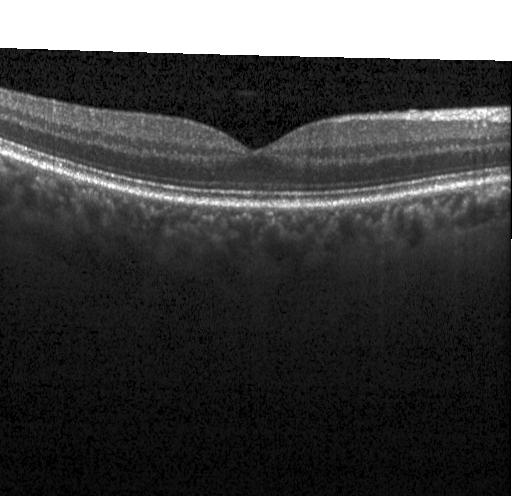 The scan shows no evidence of CNV, DME, or drusen.